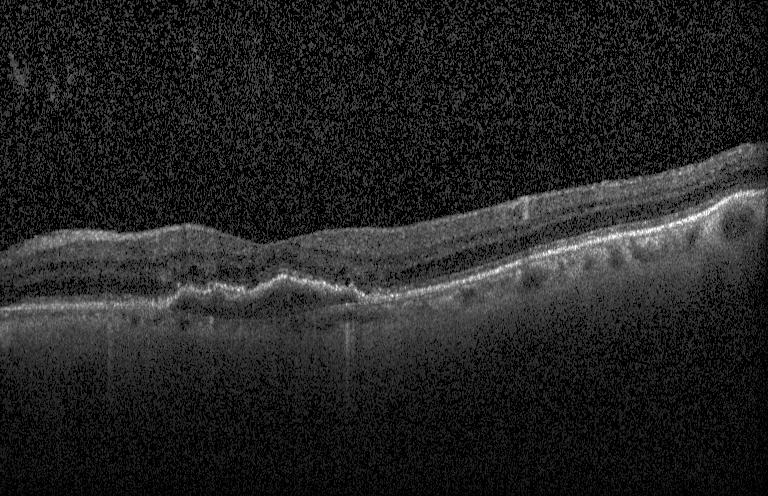 Spectral-domain OCT · retinal OCT B-scan.
CNV.